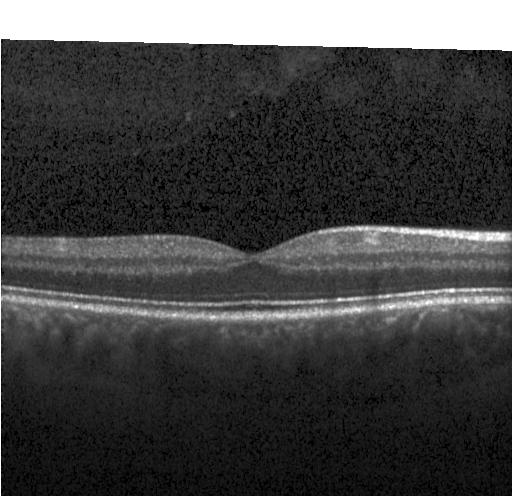 SD-OCT; OCT line scan.
Diagnosis: no choroidal neovascularization, diabetic macular edema, or drusen.